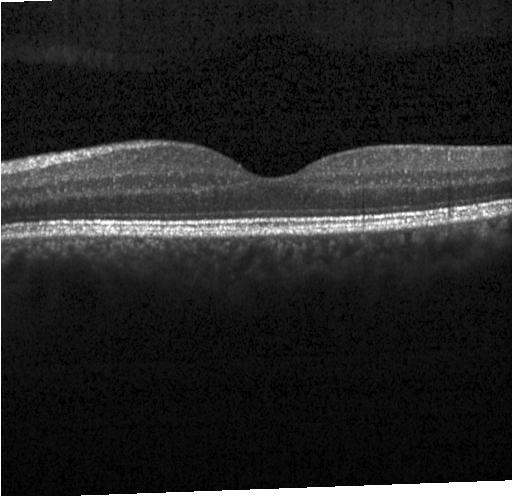 OCT line scan
This B-scan demonstrates no CNV, DME, or drusen.